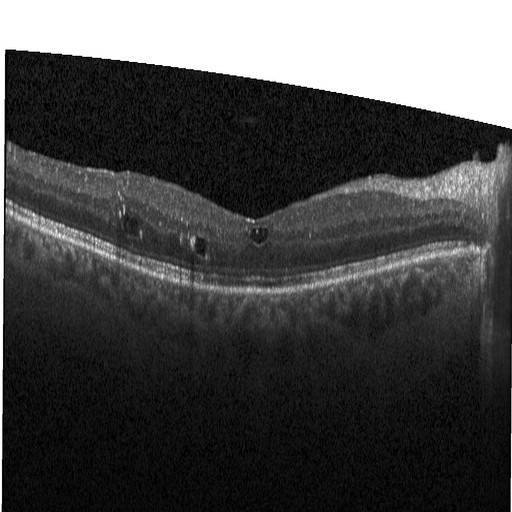 OCT line scan — The scan shows diabetic macular edema (DME).